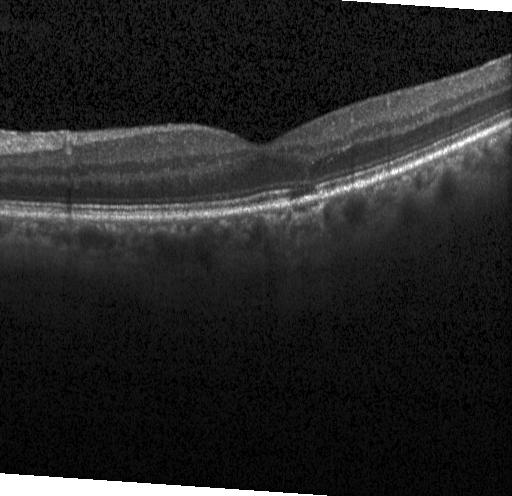 Dx: no evidence of choroidal neovascularization, diabetic macular edema, or drusen.